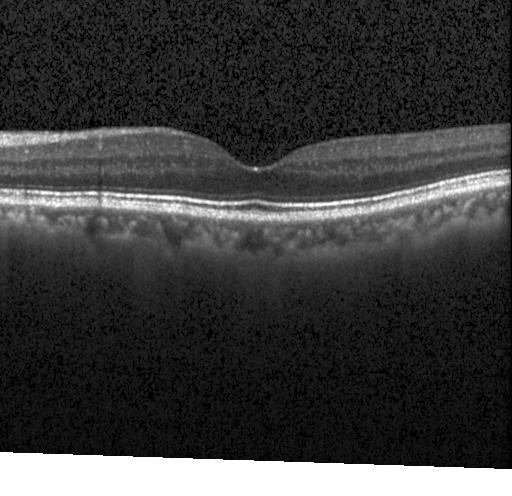

Finding: no evidence of CNV, DME, or drusen.